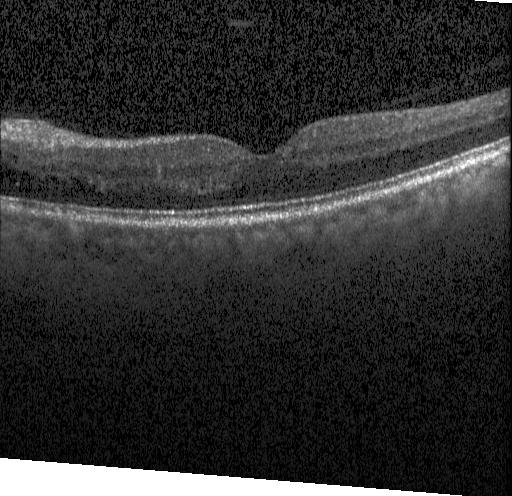
Optical coherence tomography scan · macular scan — Finding: no CNV, no DME, and no drusen.